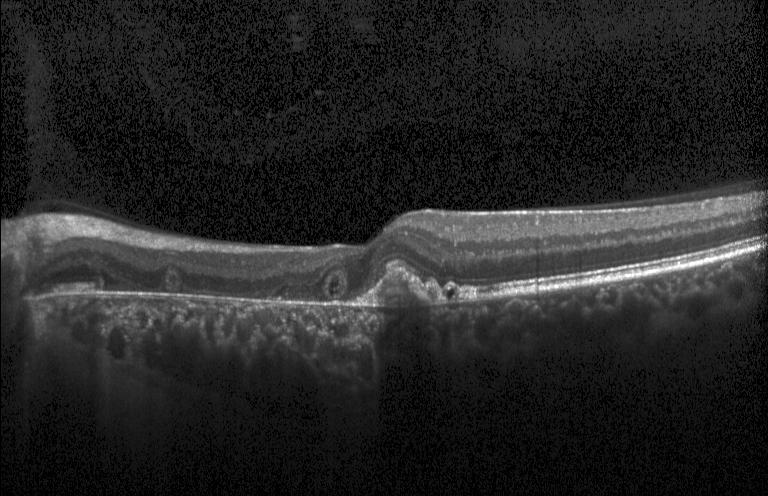
Retinal OCT B-scan · spectral-domain OCT · instrument: Heidelberg Spectralis · through the macula. Impression: a choroidal neovascular membrane.